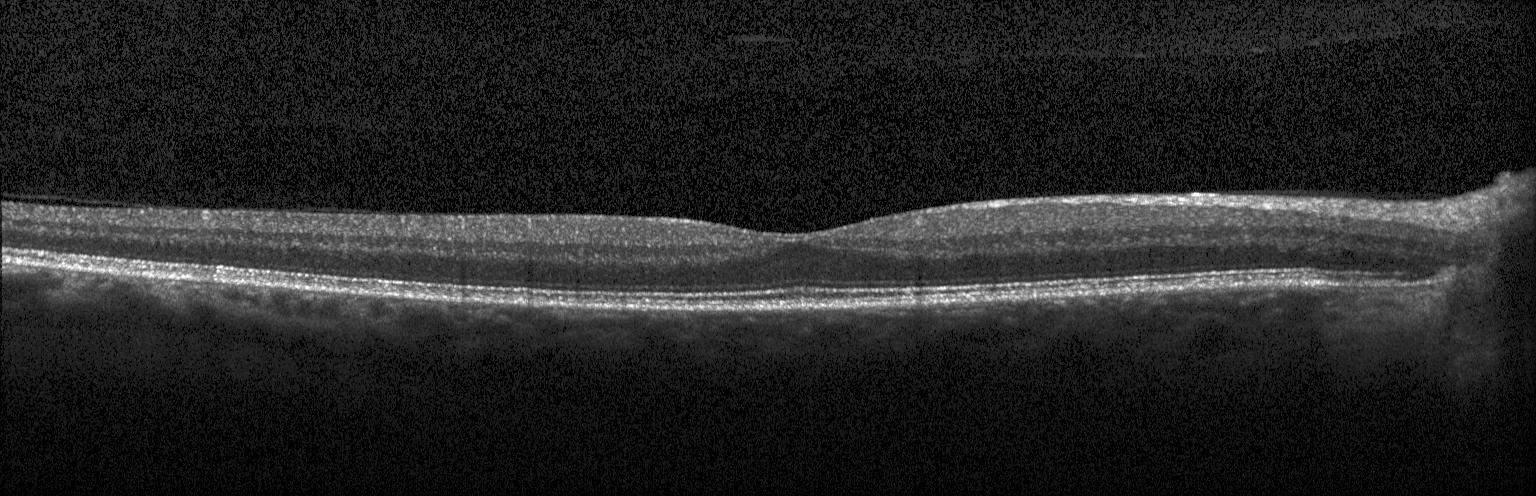 Optical coherence tomography scan
Dx: no CNV, no DME, and no drusen.